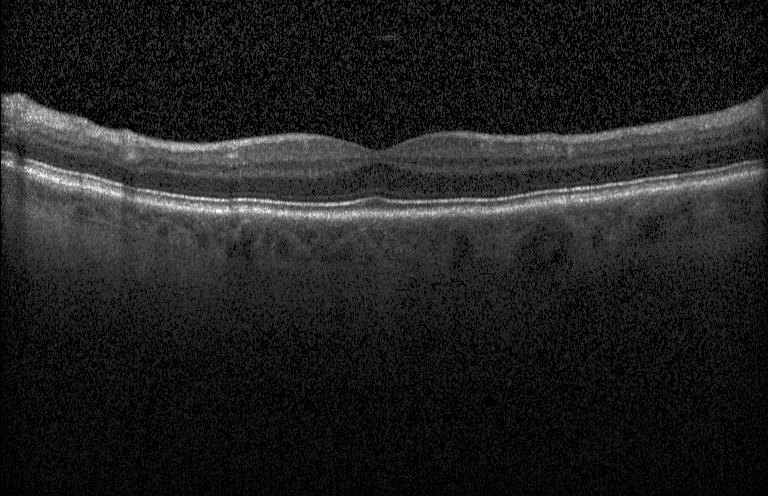
Through the macula; instrument: Heidelberg Spectralis; OCT line scan; SD-OCT — Macular OCT: no evidence of choroidal neovascularization, diabetic macular edema, or drusen.